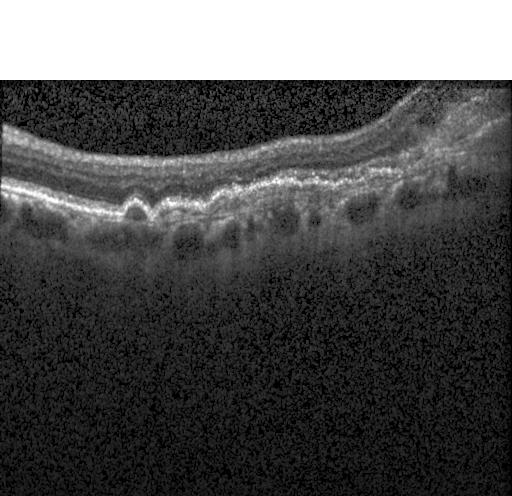
Spectral-domain optical coherence tomography · macular scan · acquired on a Heidelberg Spectralis · OCT B-scan.
Impression: choroidal neovascularization (CNV).